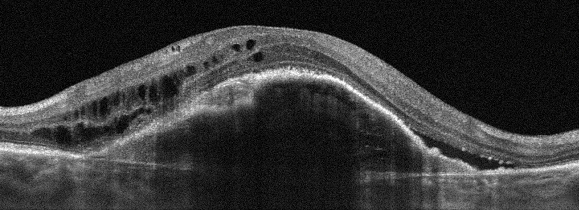
OS. Retinal OCT cross-section.
Finding: age-related macular degeneration.